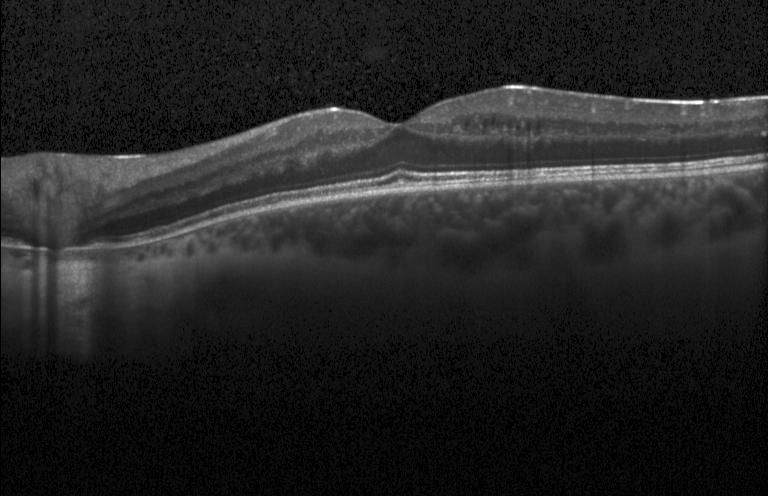
This B-scan demonstrates DME.